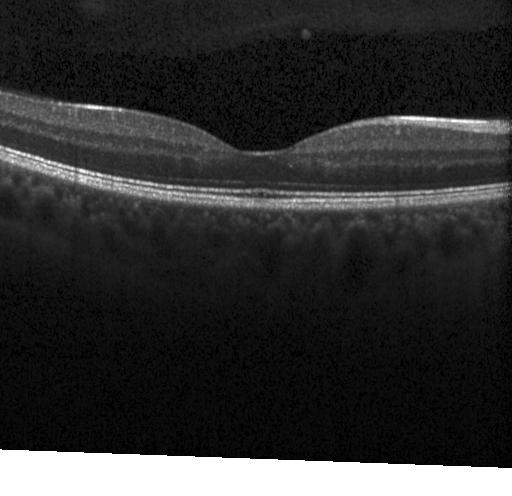
Spectral-domain OCT. OCT line scan
Diagnosis: no CNV, DME, or drusen.